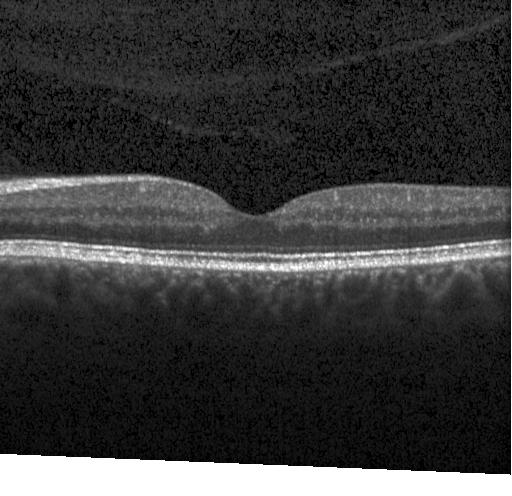 Optical coherence tomography B-scan.
Finding: neither choroidal neovascularization, diabetic macular edema, nor drusen.